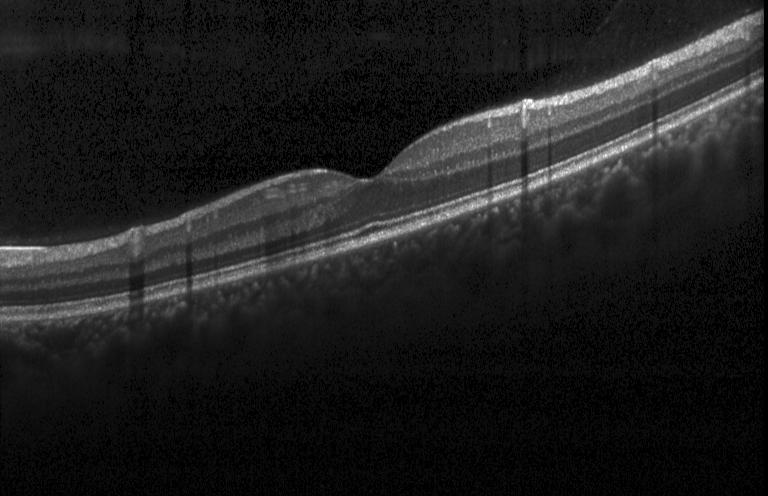 Retinal OCT cross-section
Diagnosis: no evidence of choroidal neovascularization, diabetic macular edema, or drusen.